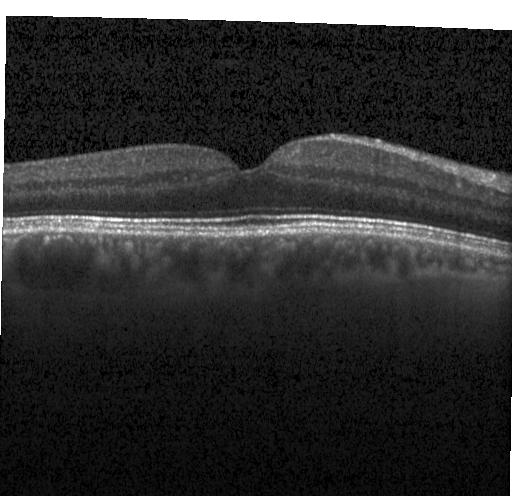

Acquired on a Heidelberg Spectralis. Macular scan. Spectral-domain optical coherence tomography. Retinal OCT cross-section
Impression: no choroidal neovascularization, diabetic macular edema, or drusen.